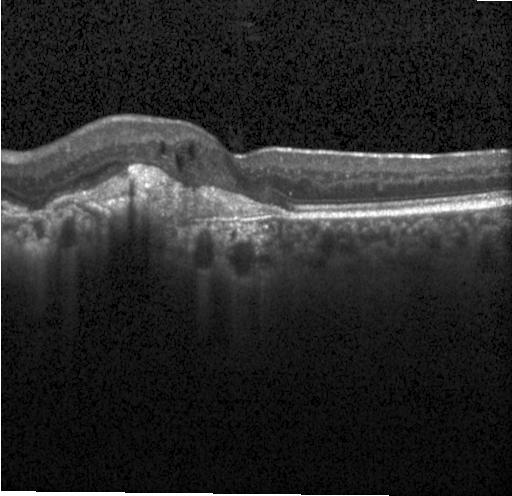 Optical coherence tomography B-scan · spectral-domain optical coherence tomography · Heidelberg Spectralis · centered on the fovea — Assessment: a choroidal neovascular membrane.